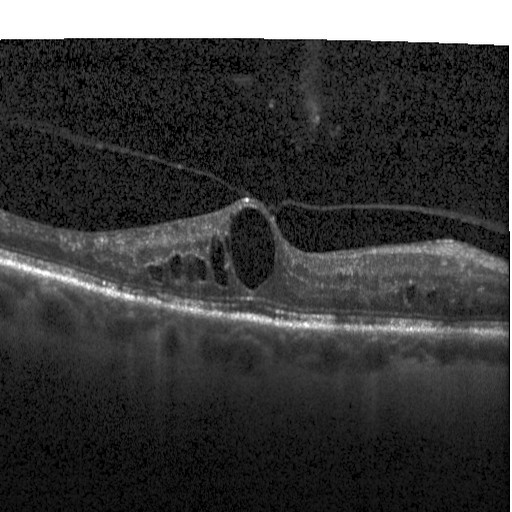
Heidelberg Spectralis OCT system. SD-OCT. Optical coherence tomography B-scan. Horizontal scan through the fovea — This B-scan demonstrates DME.